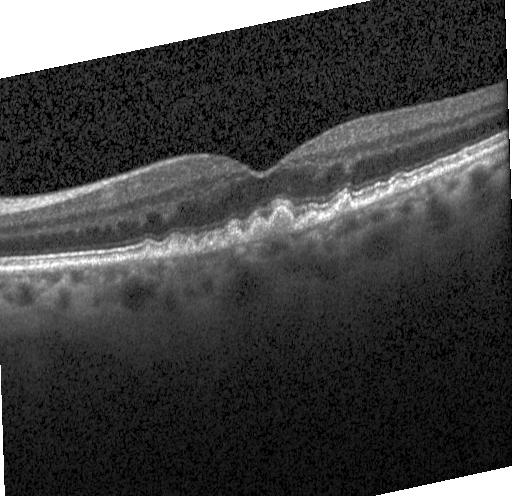

Finding: drusen.